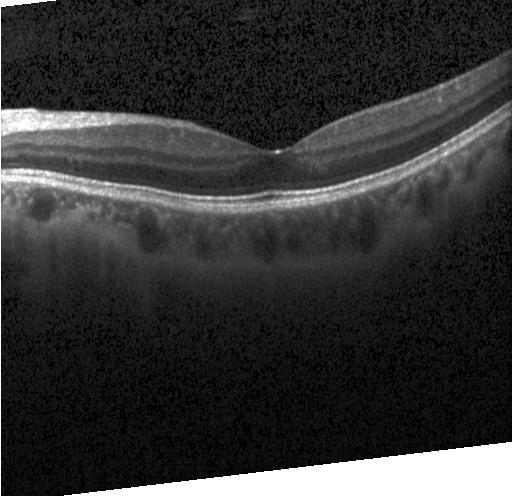 Retinal OCT cross-section · instrument: Heidelberg Spectralis
Finding: no choroidal neovascularization, diabetic macular edema, or drusen.